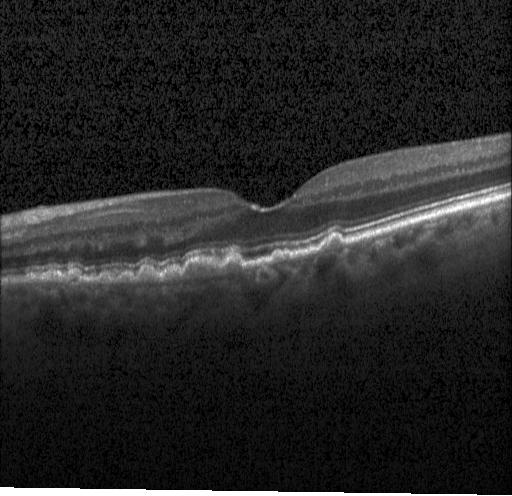 Heidelberg Spectralis OCT system; spectral-domain optical coherence tomography; OCT B-scan — The scan shows multiple drusen.